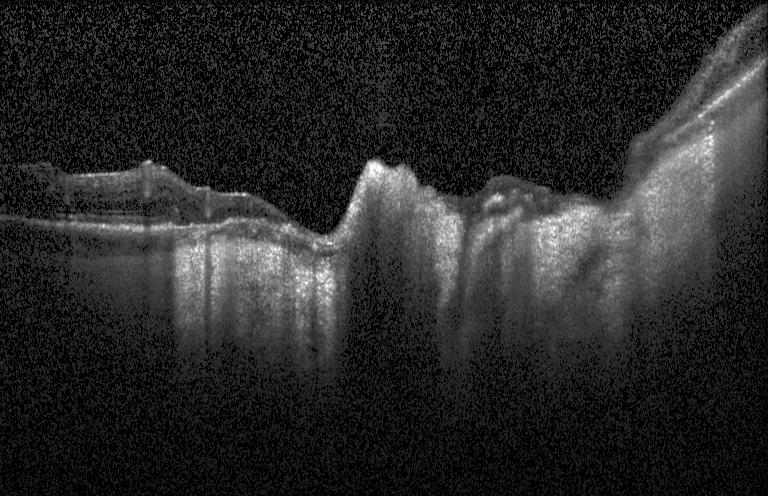

Retinal OCT B-scan — Choroidal neovascularization (CNV).